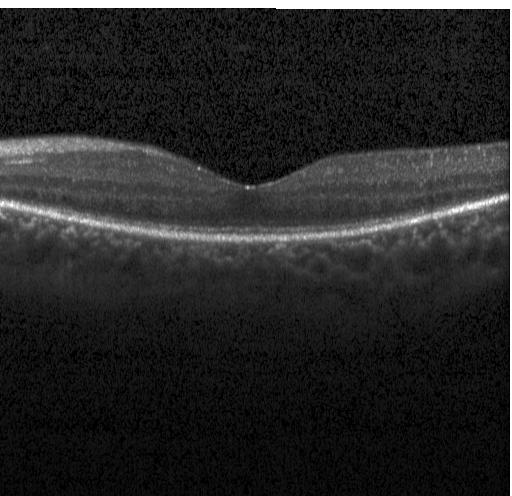

Optical coherence tomography scan — Macular OCT: no choroidal neovascularization, no diabetic macular edema, and no drusen.